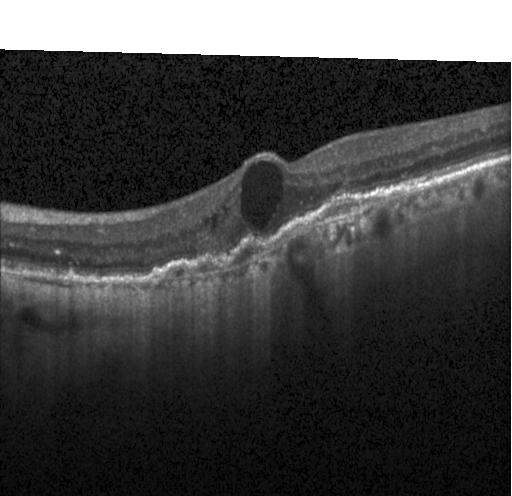

Spectral-domain optical coherence tomography. Optical coherence tomography B-scan — This B-scan demonstrates a choroidal neovascular membrane.